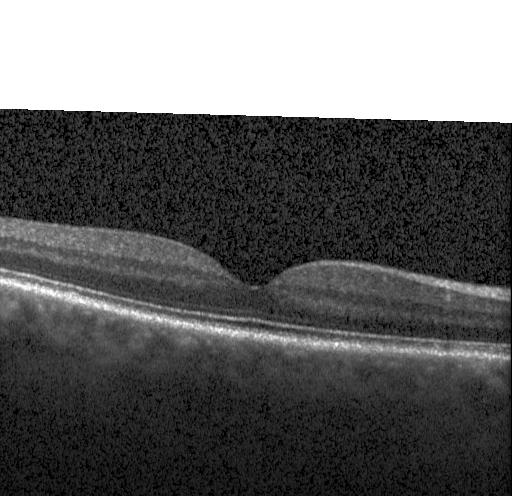

Retinal OCT cross-section showing no choroidal neovascularization, no diabetic macular edema, and no drusen.